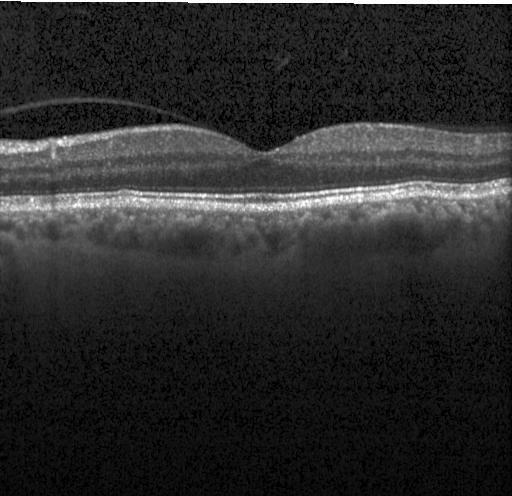

Through the macula; instrument: Heidelberg Spectralis; spectral-domain optical coherence tomography; optical coherence tomography B-scan — This B-scan demonstrates no CNV, no DME, and no drusen.